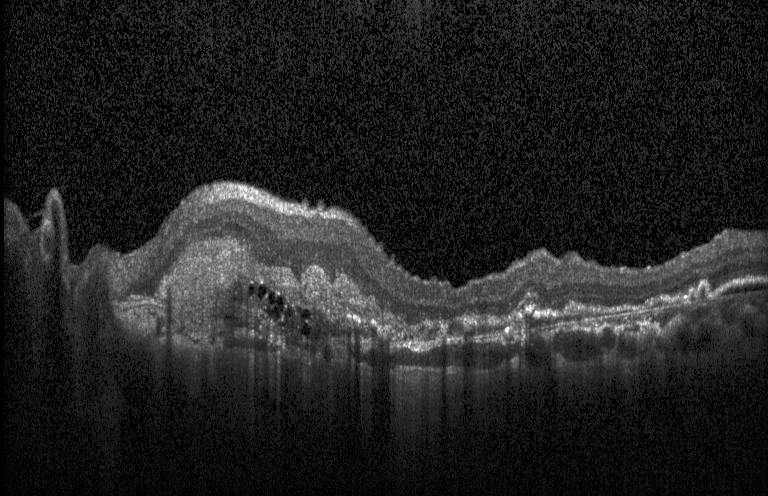
Retinal OCT B-scan · acquired on a Heidelberg Spectralis — Diagnosis: a choroidal neovascular membrane.